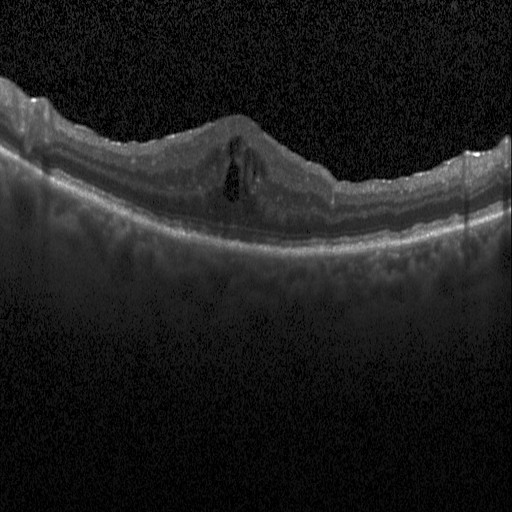

Fovea-centered · spectral-domain optical coherence tomography · Heidelberg Spectralis · retinal OCT B-scan. Macular OCT: DME.